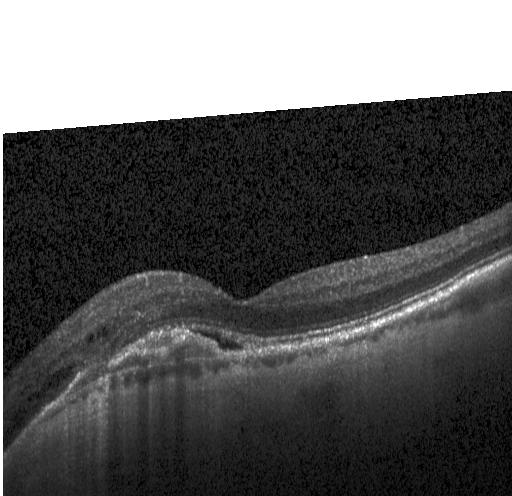 Heidelberg Spectralis, optical coherence tomography scan, macular scan
Diagnosis: choroidal neovascularization.